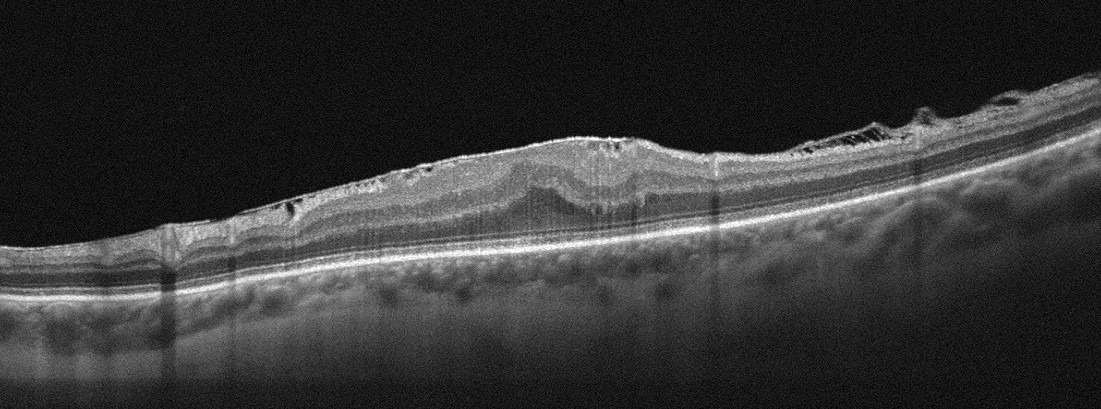 Optical coherence tomography scan. Optovue Avanti RTVue XR. Fovea-centered.
Diagnosis: epiretinal membrane.